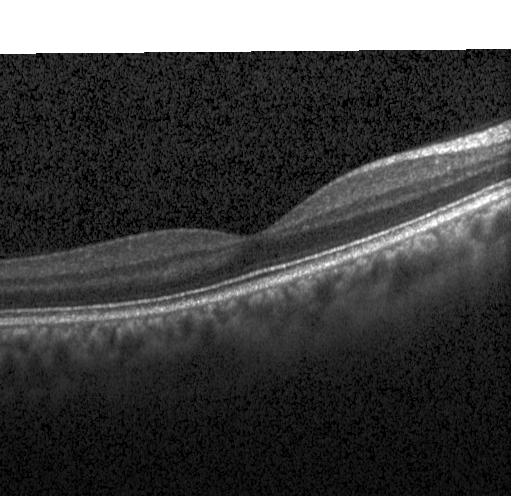
Spectral-domain OCT B-scan: no CNV, no DME, and no drusen.